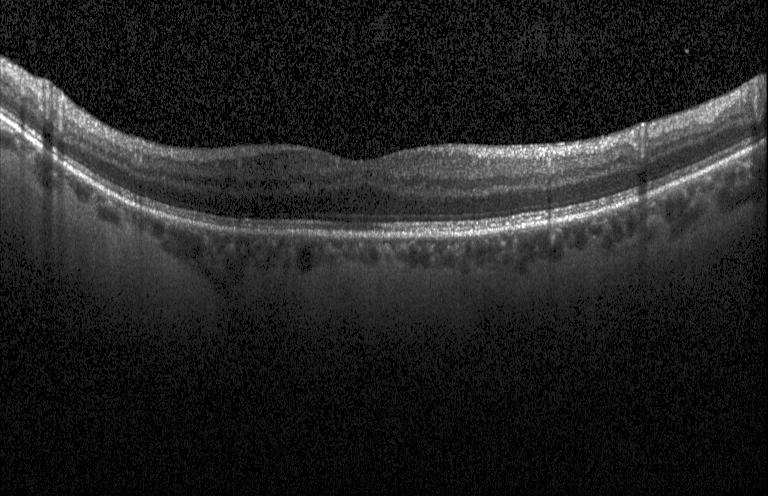

Retinal OCT B-scan, spectral-domain optical coherence tomography. Diagnosis: no choroidal neovascularization, diabetic macular edema, or drusen.